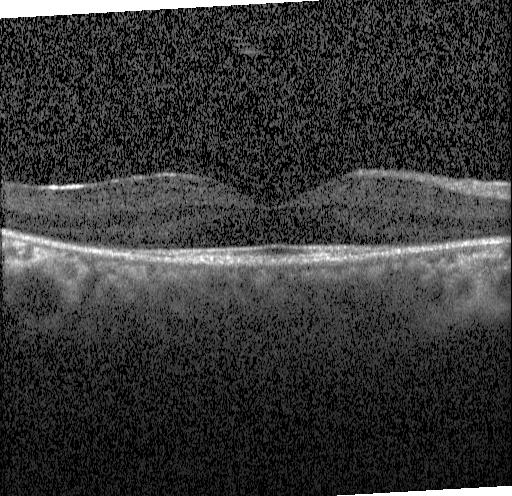

Spectral-domain optical coherence tomography · optical coherence tomography scan. Diagnosis: no choroidal neovascularization, diabetic macular edema, or drusen.